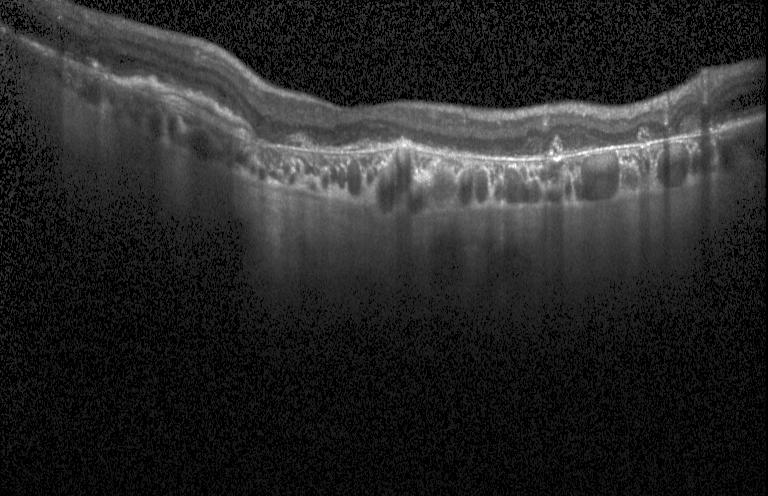
Diagnosis: CNV.